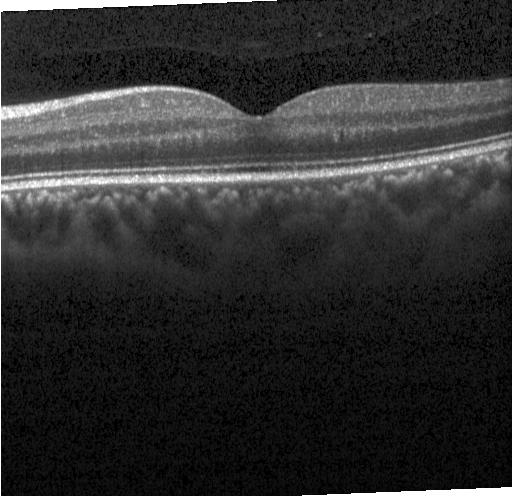

SD-OCT. Optical coherence tomography B-scan — The scan shows no CNV, no DME, and no drusen.